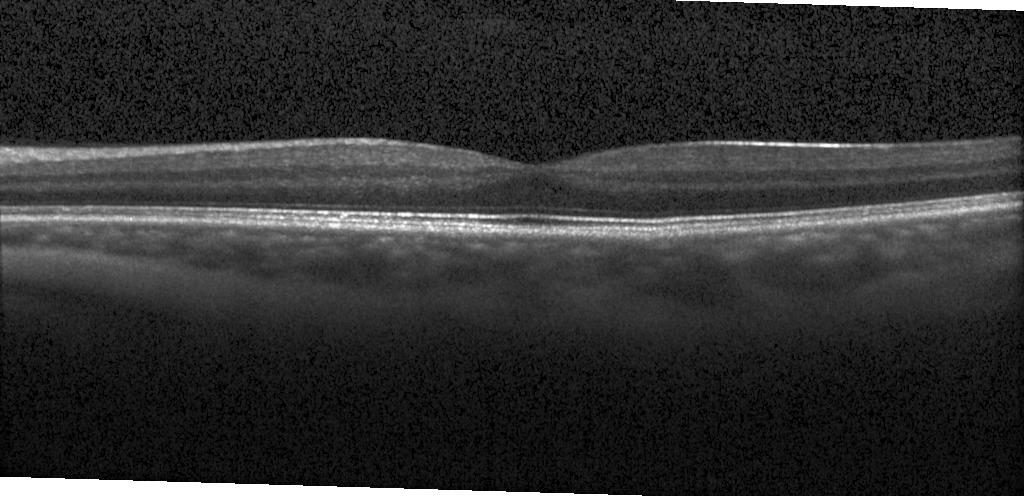 Macular OCT: neither choroidal neovascularization, diabetic macular edema, nor drusen.